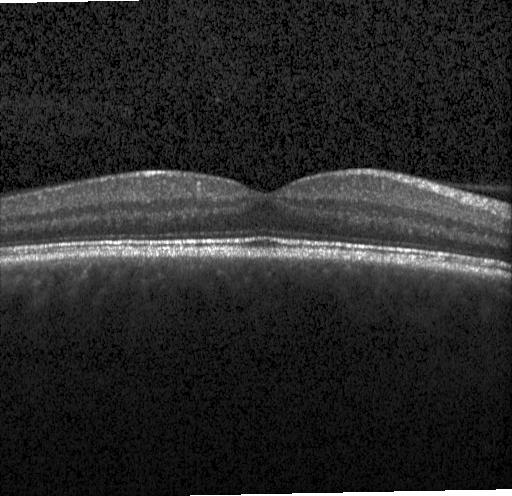
Impression: no choroidal neovascularization, no diabetic macular edema, and no drusen.